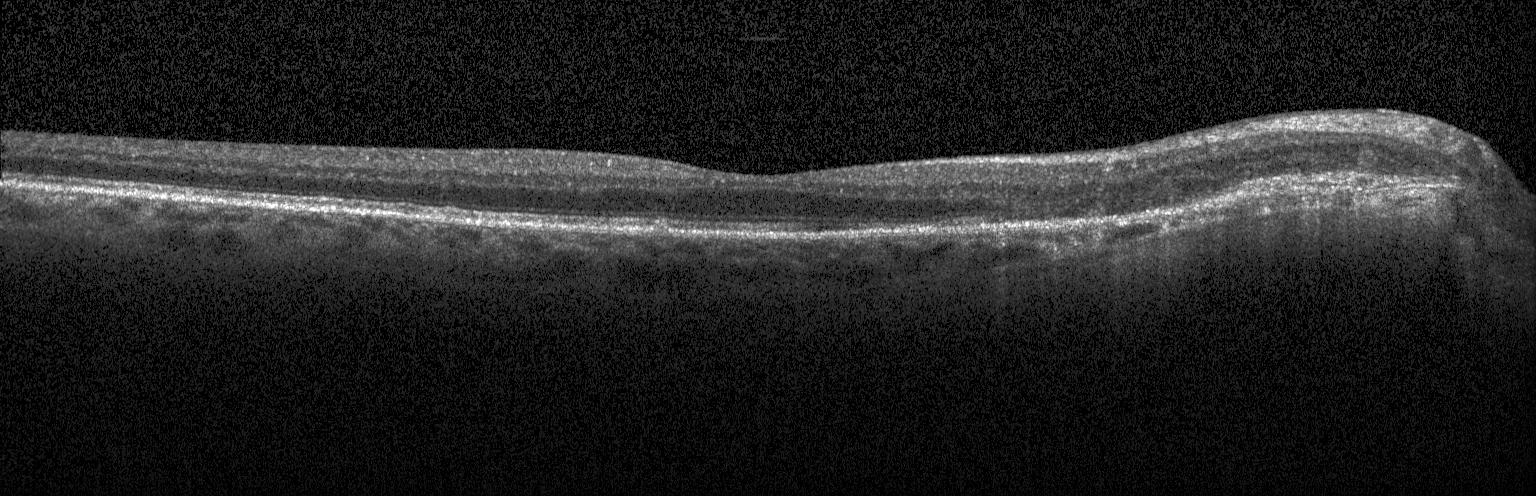
Dx: a choroidal neovascular membrane.